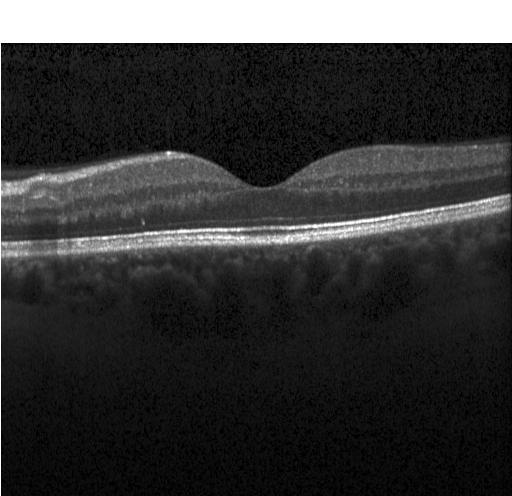

Spectral-domain OCT · retinal OCT cross-section · instrument: Heidelberg Spectralis
Neither choroidal neovascularization, diabetic macular edema, nor drusen.